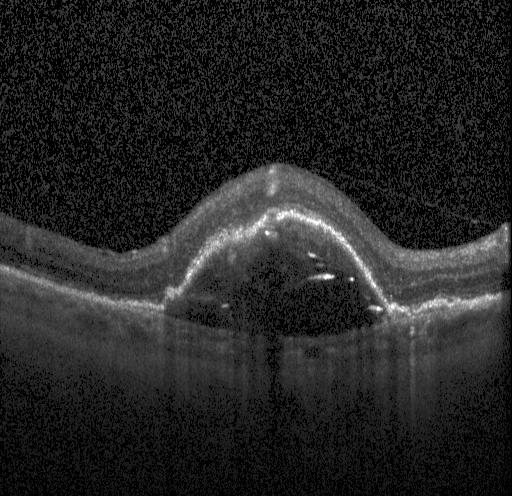

Retinal OCT cross-section · Heidelberg Spectralis OCT system · fovea-centered · SD-OCT — CNV.